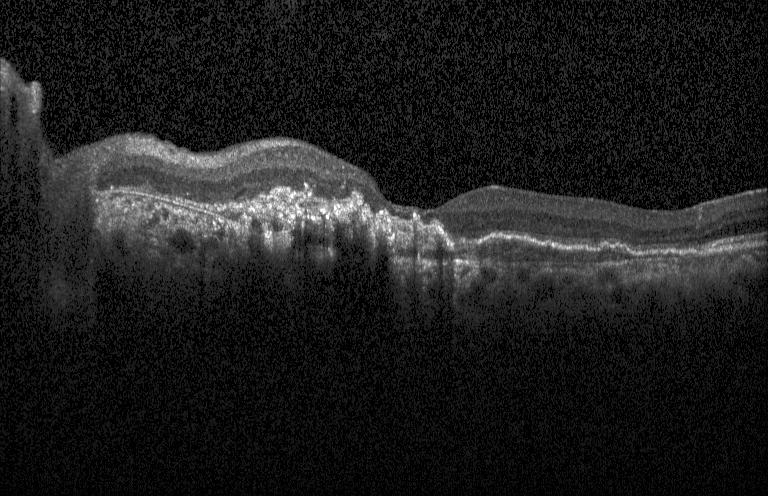 Dx: choroidal neovascularization.